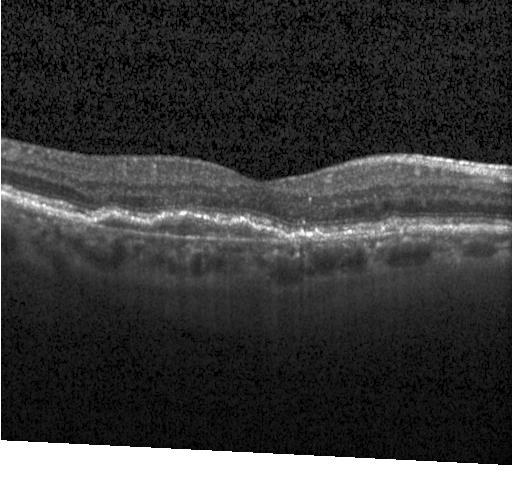

Optical coherence tomography scan. Acquired on a Heidelberg Spectralis
Macular OCT: a choroidal neovascular membrane.